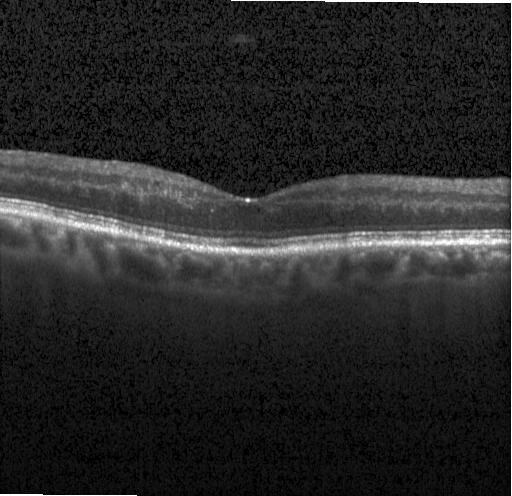 Diagnosis: no choroidal neovascularization, diabetic macular edema, or drusen.